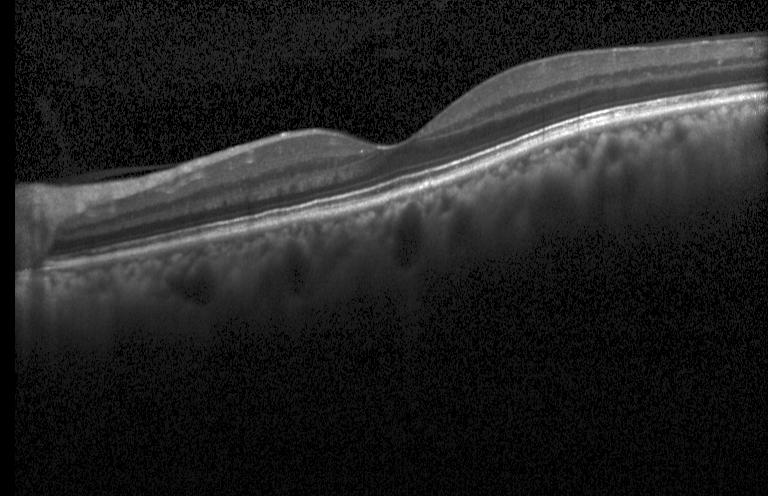
This B-scan demonstrates no choroidal neovascularization, diabetic macular edema, or drusen.